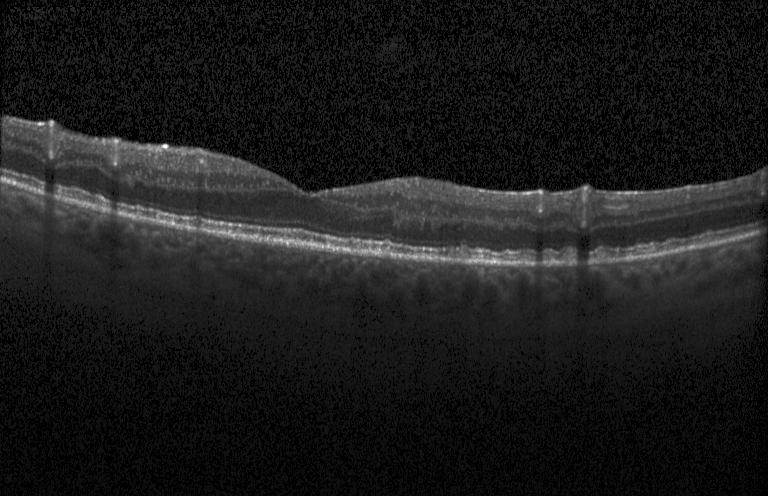 Finding: no choroidal neovascularization, diabetic macular edema, or drusen.